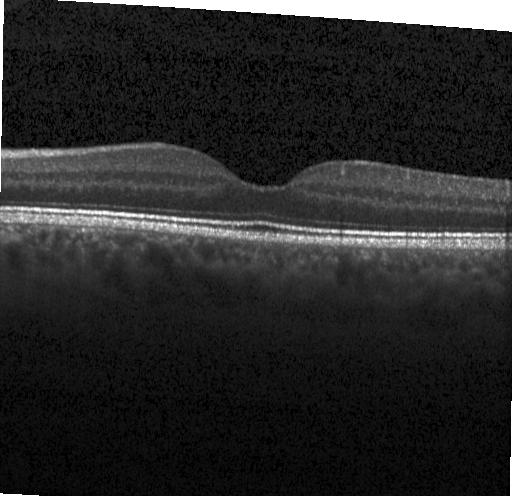
OCT line scan.
This B-scan demonstrates no choroidal neovascularization, no diabetic macular edema, and no drusen.